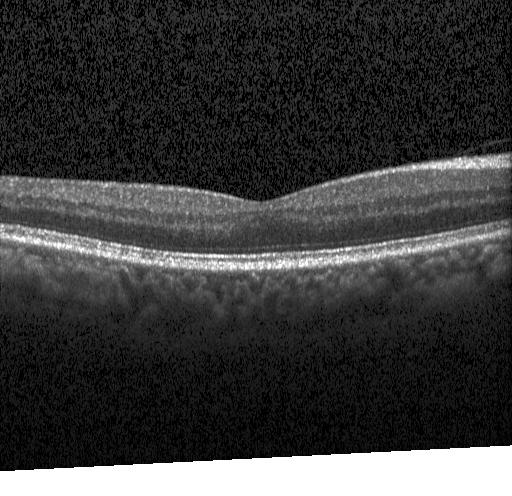

Instrument: Heidelberg Spectralis · centered on the fovea · spectral-domain OCT · optical coherence tomography scan — Dx: neither CNV, DME, nor drusen.